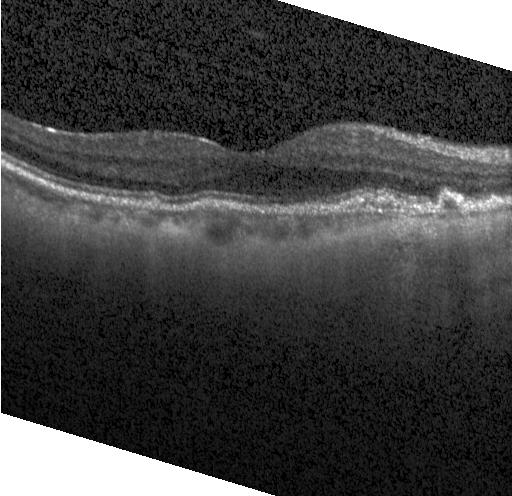

OCT line scan. Spectral-domain OCT. This B-scan demonstrates drusen.